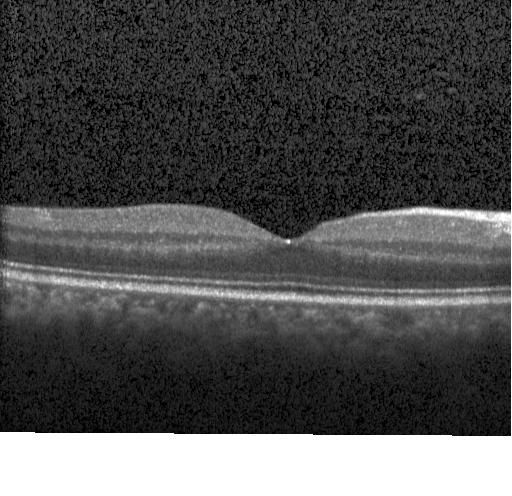 Acquired on a Heidelberg Spectralis. Fovea-centered. Spectral-domain OCT. Optical coherence tomography B-scan
Finding: no evidence of choroidal neovascularization, diabetic macular edema, or drusen.